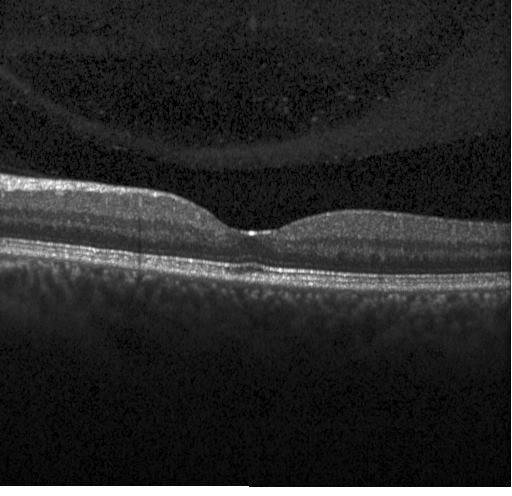 Through the macula. OCT line scan
Diagnosis: no choroidal neovascularization, no diabetic macular edema, and no drusen.